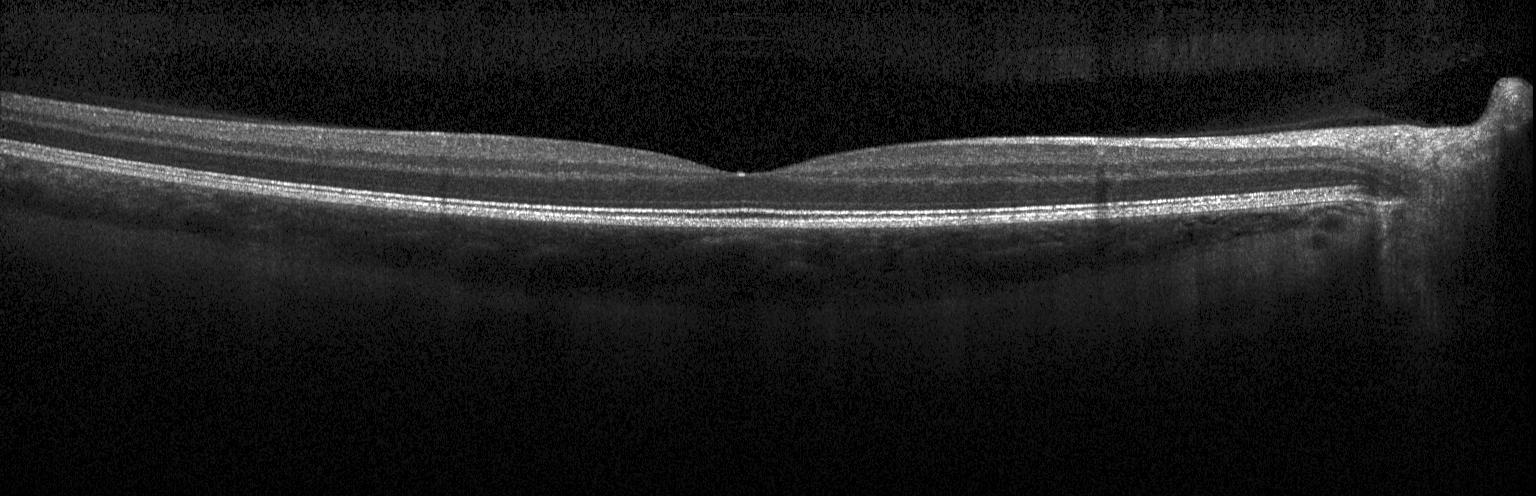

OCT finding: no evidence of CNV, DME, or drusen.